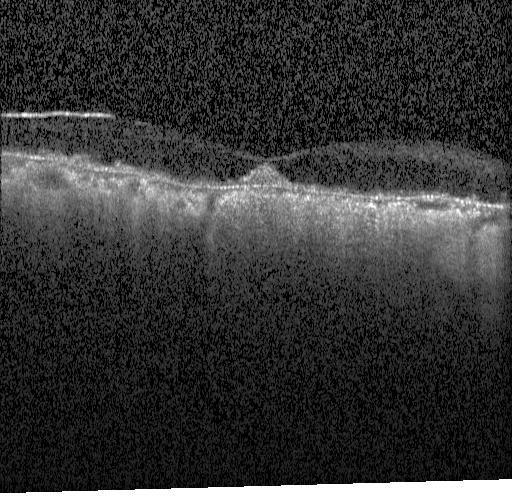
Diagnosis: a choroidal neovascular membrane.